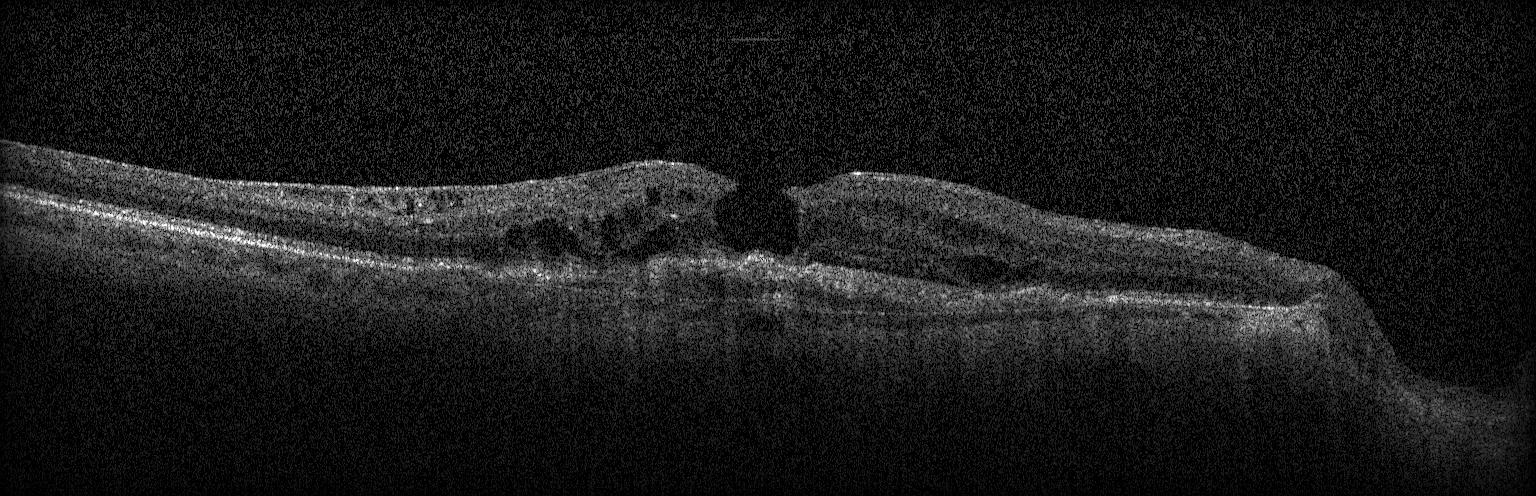 This B-scan demonstrates a choroidal neovascular membrane.